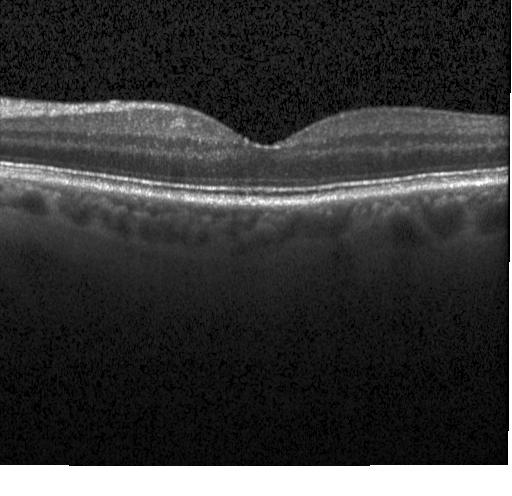 Retinal OCT B-scan.
Diagnosis: neither choroidal neovascularization, diabetic macular edema, nor drusen.